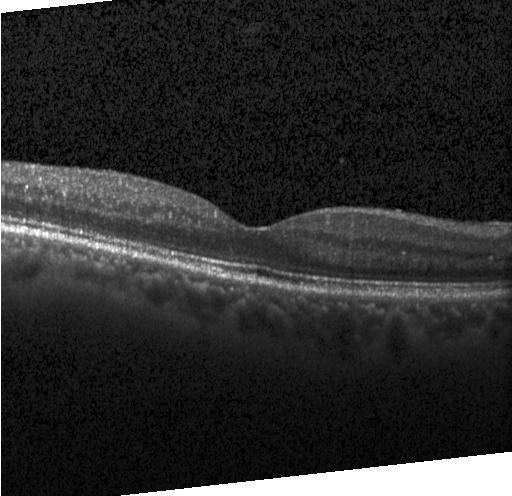
Spectral-domain OCT · acquired on a Heidelberg Spectralis · OCT B-scan · horizontal scan through the fovea — Dx: no evidence of choroidal neovascularization, diabetic macular edema, or drusen.